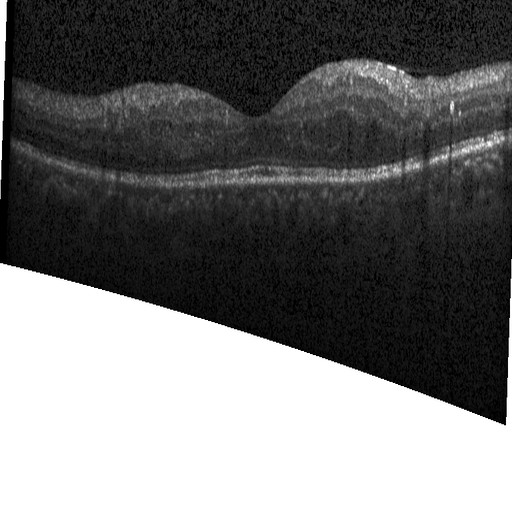 Through the macula. Retinal OCT B-scan. SD-OCT. Heidelberg Spectralis OCT system — OCT finding: DME.